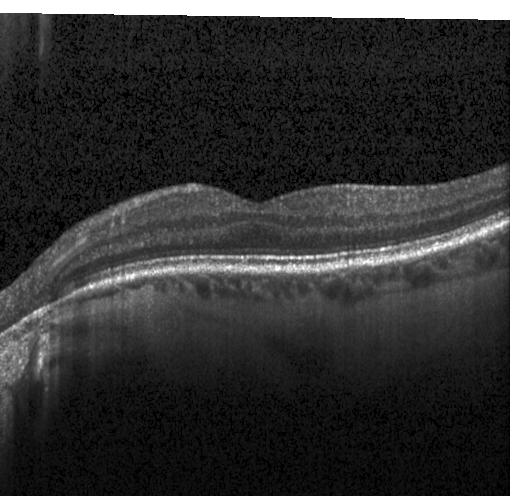
Optical coherence tomography scan · through the macula.
Impression: neither choroidal neovascularization, diabetic macular edema, nor drusen.